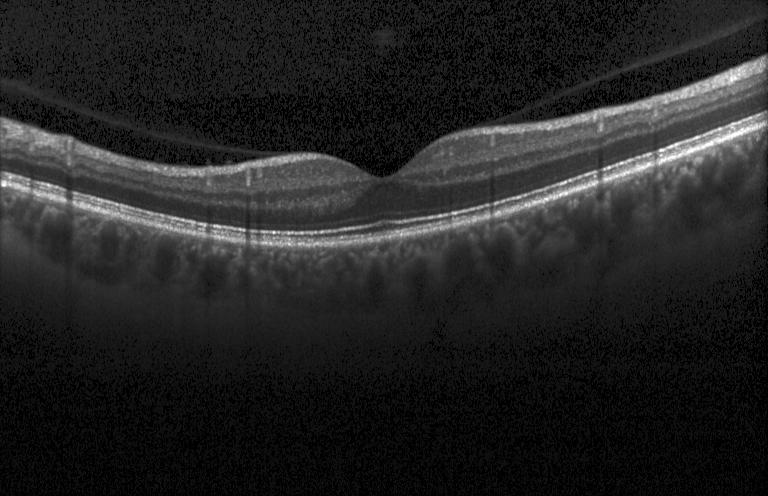
Retinal OCT cross-section · fovea-centered · instrument: Heidelberg Spectralis. Assessment: no evidence of CNV, DME, or drusen.